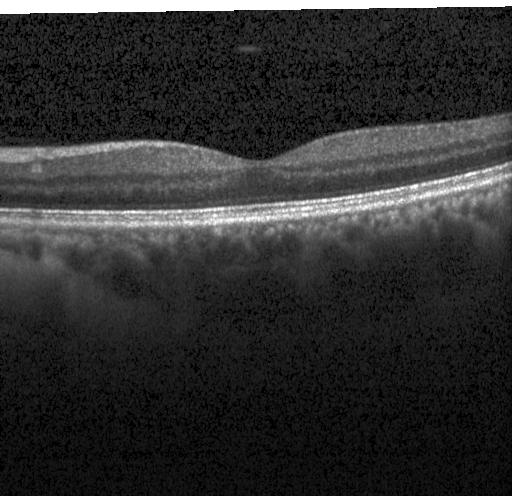
Acquired on a Heidelberg Spectralis; spectral-domain OCT; optical coherence tomography B-scan. Diagnosis: no CNV, no DME, and no drusen.